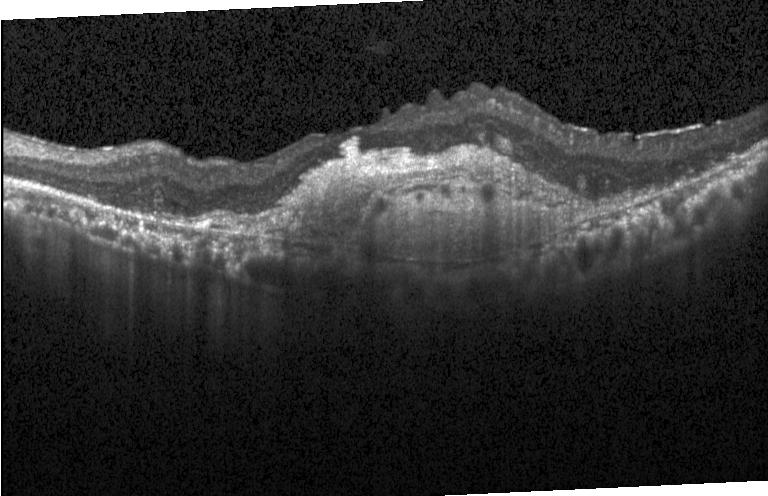

SD-OCT, optical coherence tomography scan
A choroidal neovascular membrane.